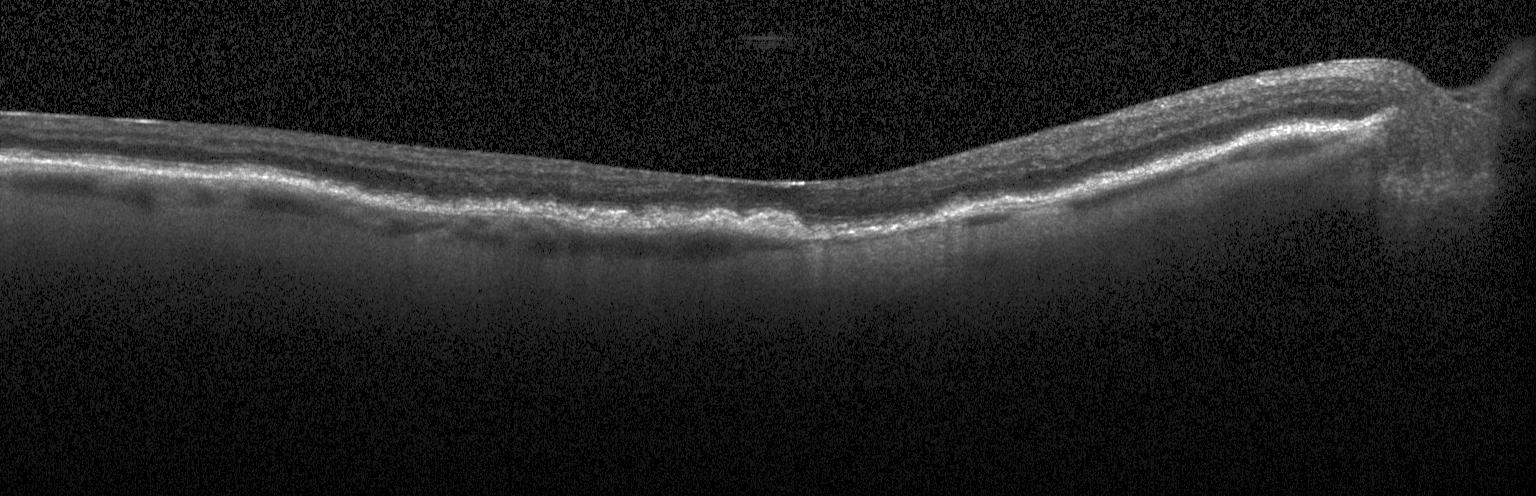
OCT B-scan showing a choroidal neovascular membrane.